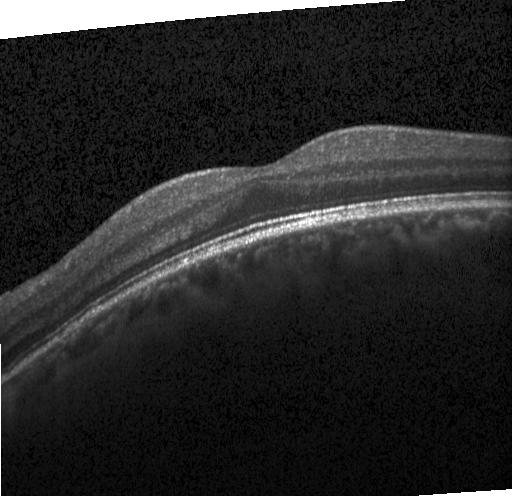
Instrument: Heidelberg Spectralis · centered on the fovea · retinal OCT B-scan — Assessment: no evidence of choroidal neovascularization, diabetic macular edema, or drusen.